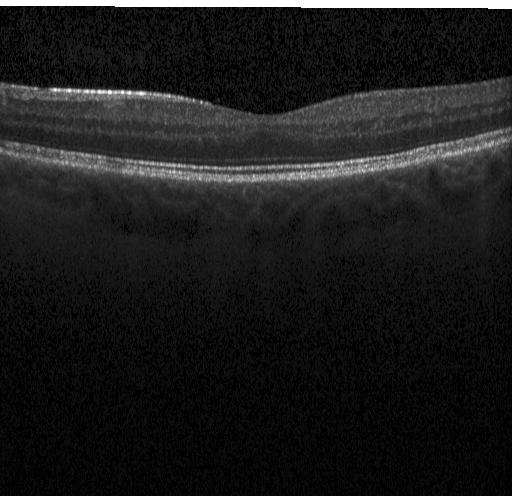
Finding: neither choroidal neovascularization, diabetic macular edema, nor drusen.